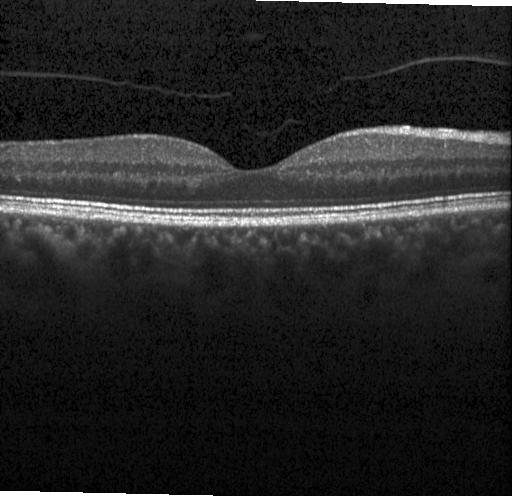

The scan shows no choroidal neovascularization, no diabetic macular edema, and no drusen.